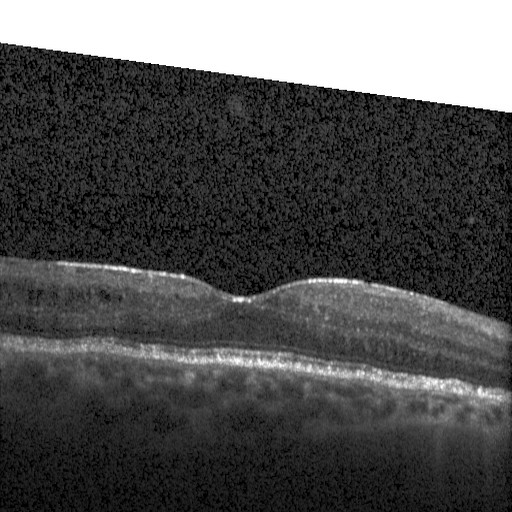
Acquired on a Heidelberg Spectralis. SD-OCT. Optical coherence tomography B-scan.
The scan shows diabetic macular edema (DME).